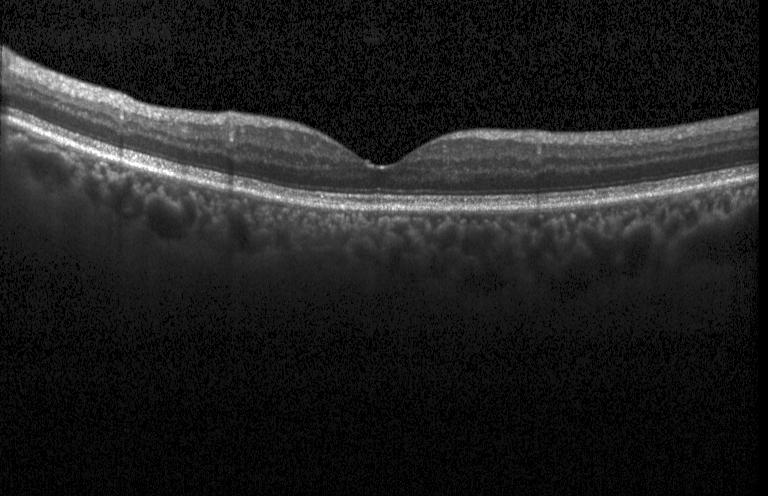 Spectral-domain OCT. Retinal OCT B-scan. Acquired on a Heidelberg Spectralis
Finding: no evidence of choroidal neovascularization, diabetic macular edema, or drusen.